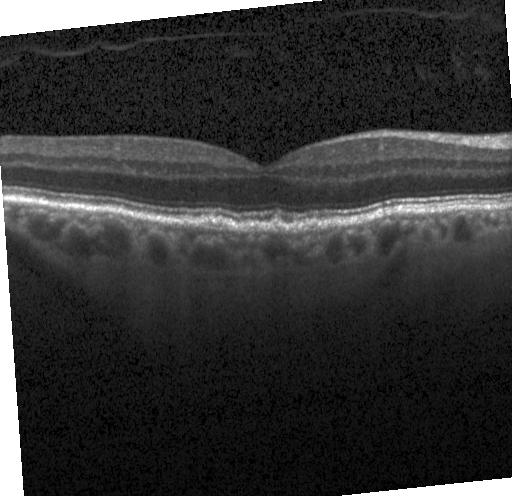 Retinal OCT B-scan, Heidelberg Spectralis — This B-scan demonstrates multiple drusen.